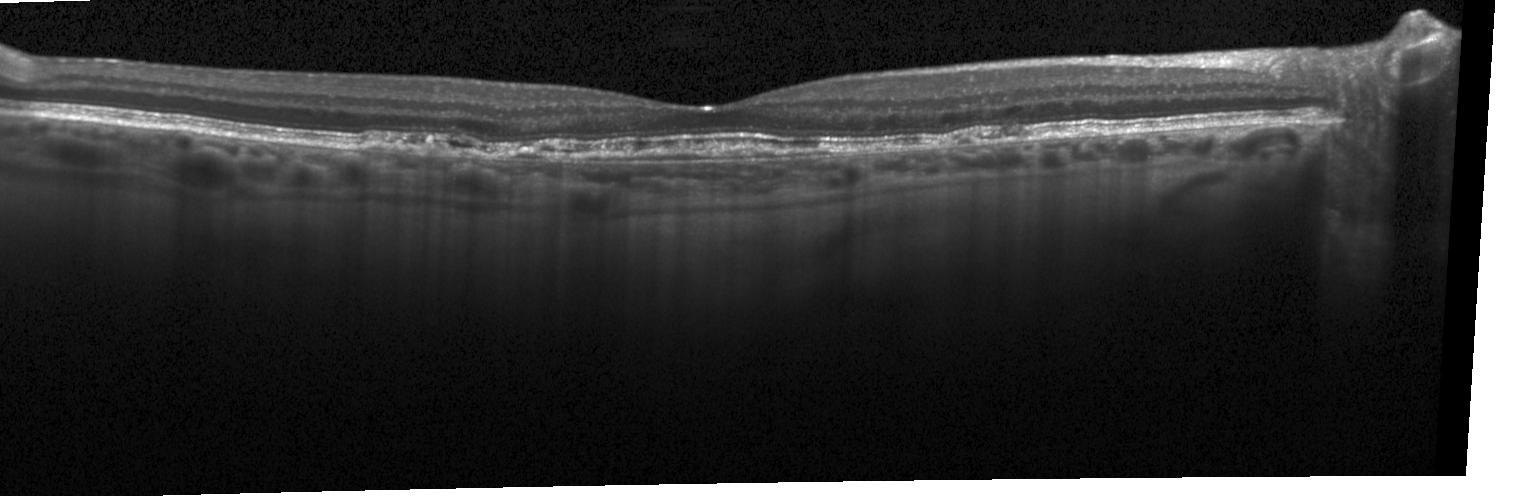

A choroidal neovascular membrane.